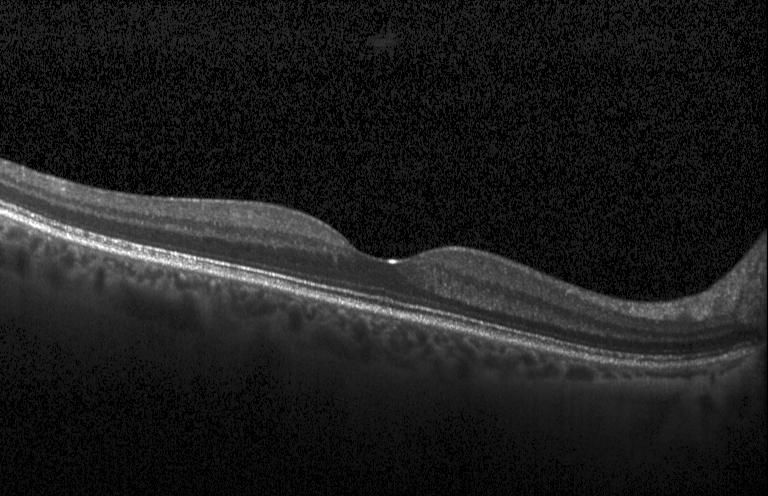

Acquired on a Heidelberg Spectralis; through the macula; spectral-domain OCT; OCT B-scan. OCT finding: no choroidal neovascularization, diabetic macular edema, or drusen.